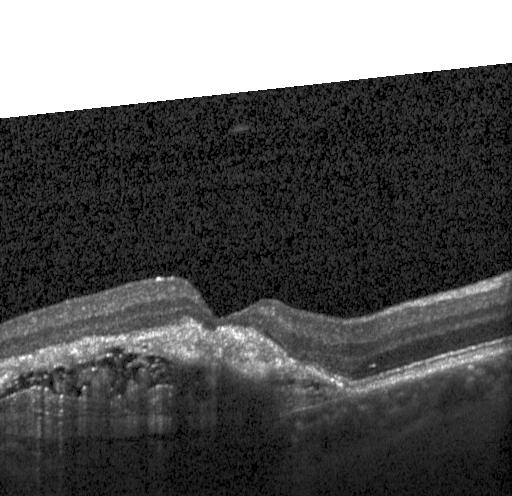
OCT line scan — Diagnosis: choroidal neovascularization (CNV).